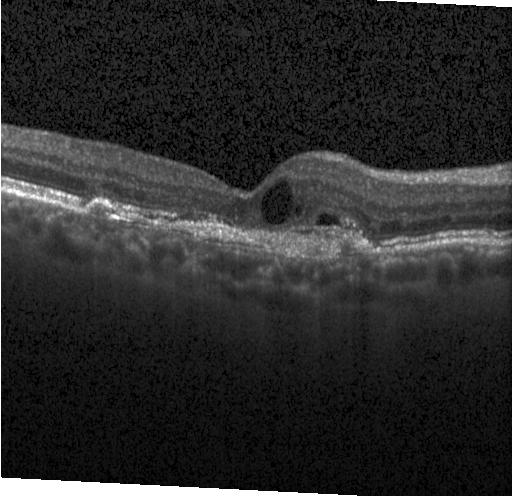

Fovea-centered; OCT line scan; acquired on a Heidelberg Spectralis; spectral-domain optical coherence tomography
Assessment: a choroidal neovascular membrane.